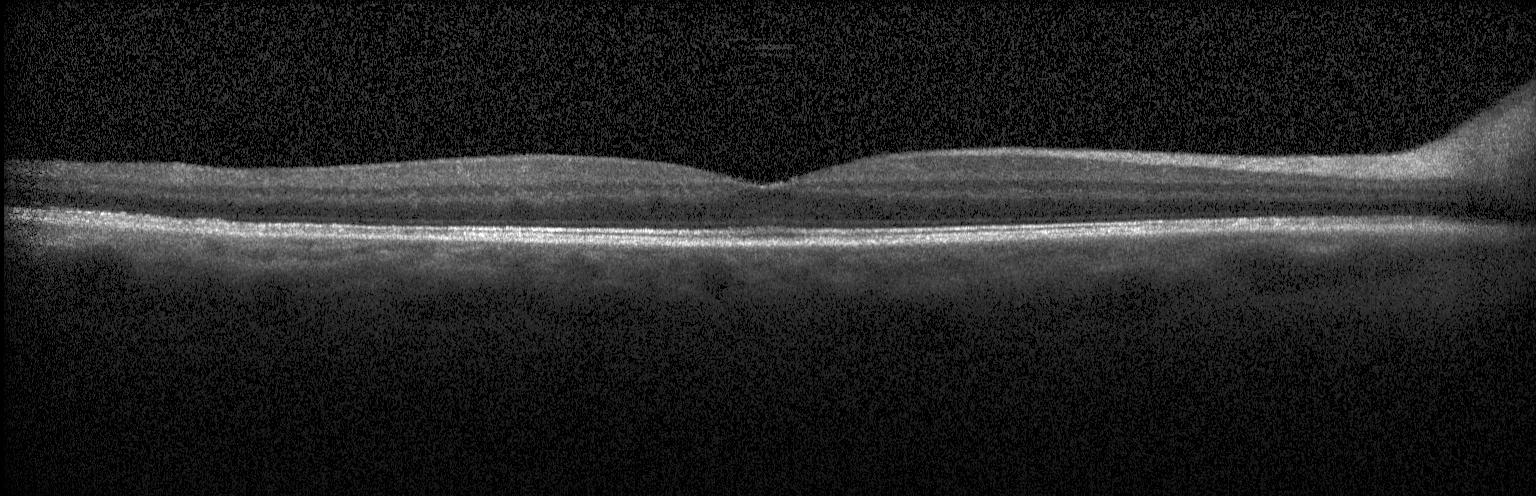
Optical coherence tomography scan
Diagnosis: neither CNV, DME, nor drusen.